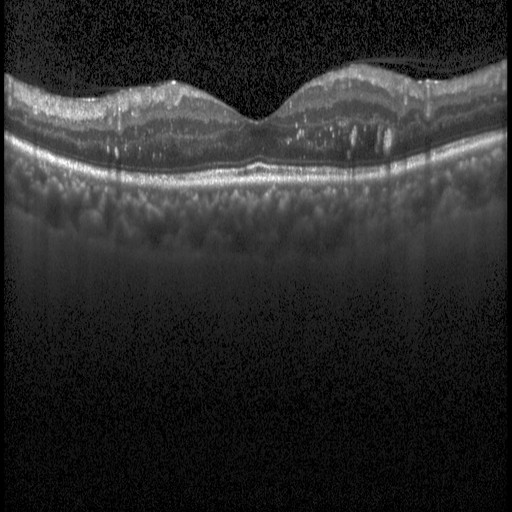

Optical coherence tomography scan
This B-scan demonstrates diabetic macular edema.